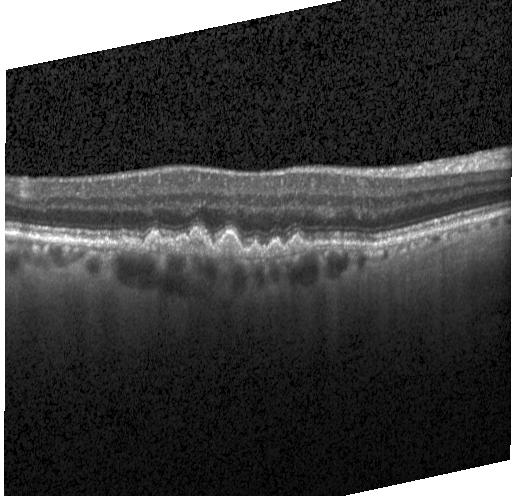
Spectral-domain OCT. Heidelberg Spectralis OCT system. Macular scan. Optical coherence tomography B-scan
Impression: drusen.